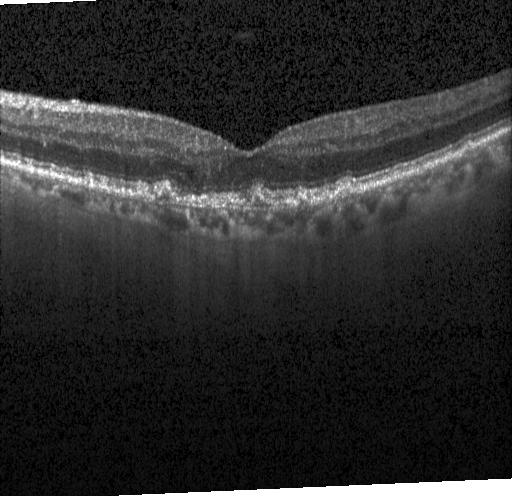
Centered on the fovea. Spectral-domain optical coherence tomography. OCT B-scan.
Impression: multiple drusen.